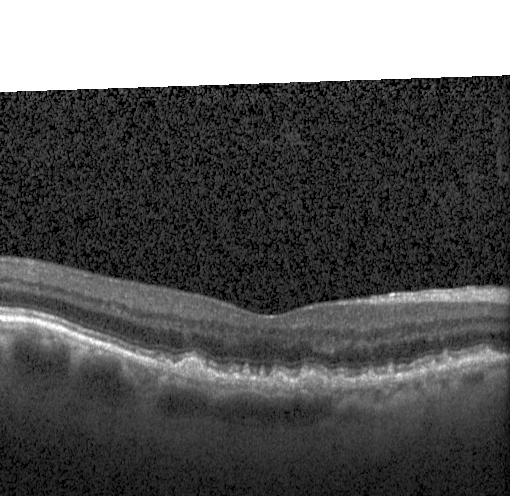

OCT B-scan — OCT finding: sub-RPE drusenoid deposits.